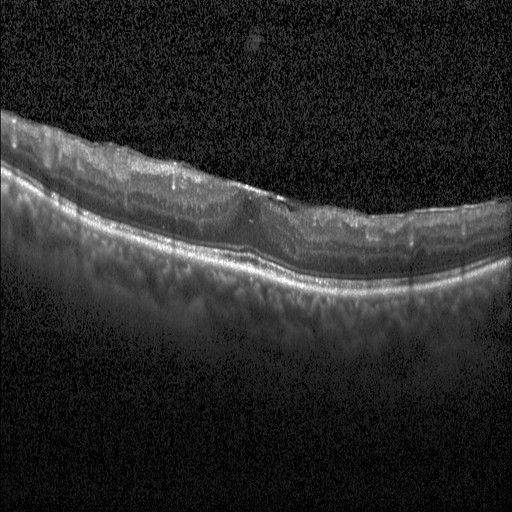 OCT finding: diabetic macular edema.